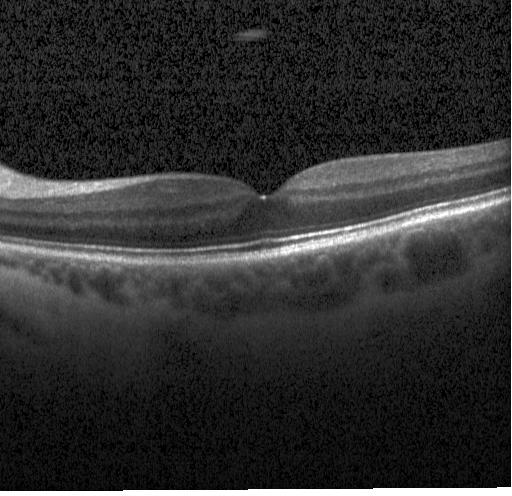 OCT B-scan · macular scan · SD-OCT.
Impression: no evidence of choroidal neovascularization, diabetic macular edema, or drusen.